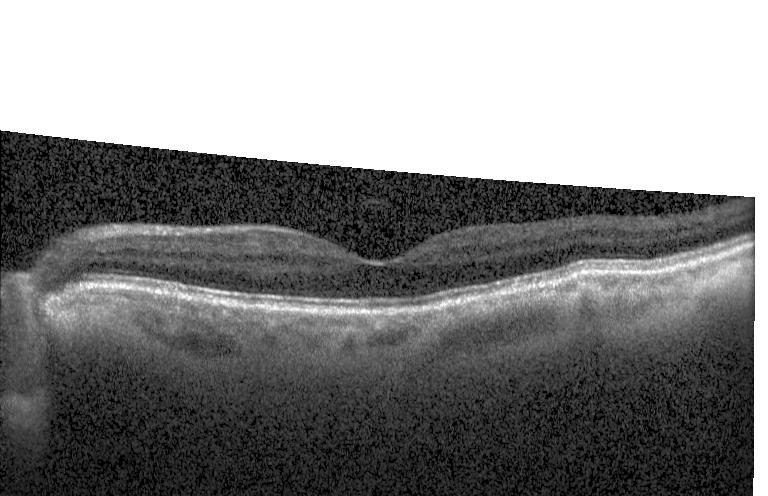
Instrument: Heidelberg Spectralis · retinal OCT cross-section.
This B-scan demonstrates no choroidal neovascularization, no diabetic macular edema, and no drusen.